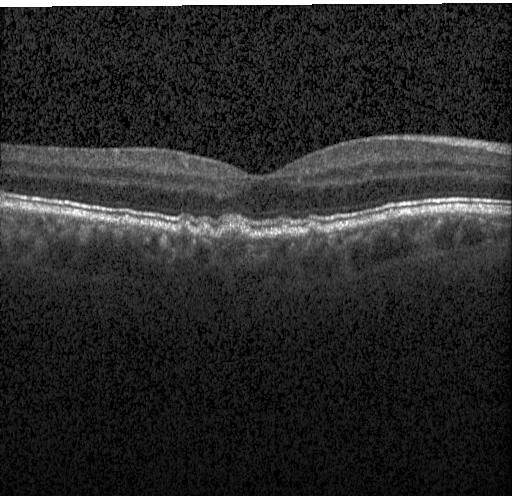

Retinal OCT cross-section · fovea-centered · instrument: Heidelberg Spectralis. Diagnosis: multiple drusen.